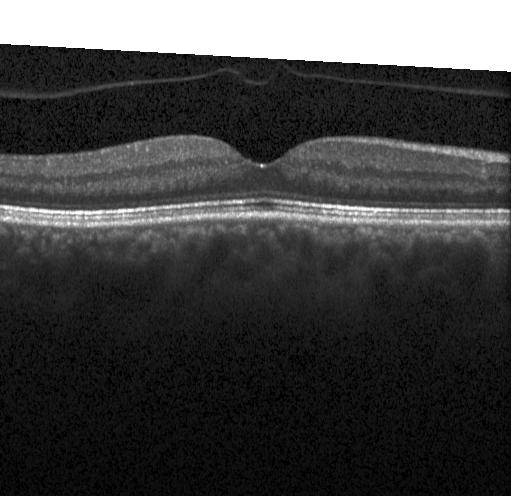

Spectral-domain optical coherence tomography, retinal OCT B-scan. The scan shows neither choroidal neovascularization, diabetic macular edema, nor drusen.